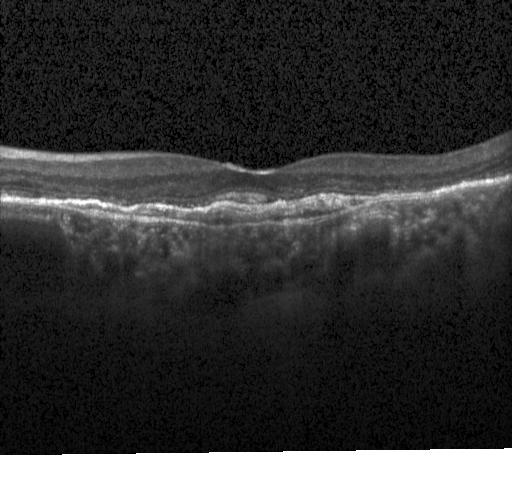
Retinal OCT B-scan.
Diagnosis: a choroidal neovascular membrane.